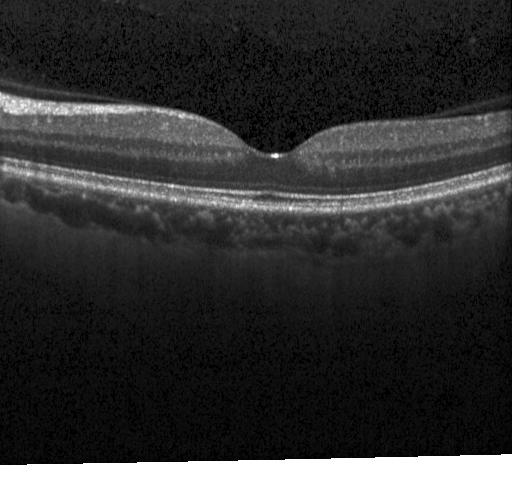
Diagnosis: no choroidal neovascularization, diabetic macular edema, or drusen.